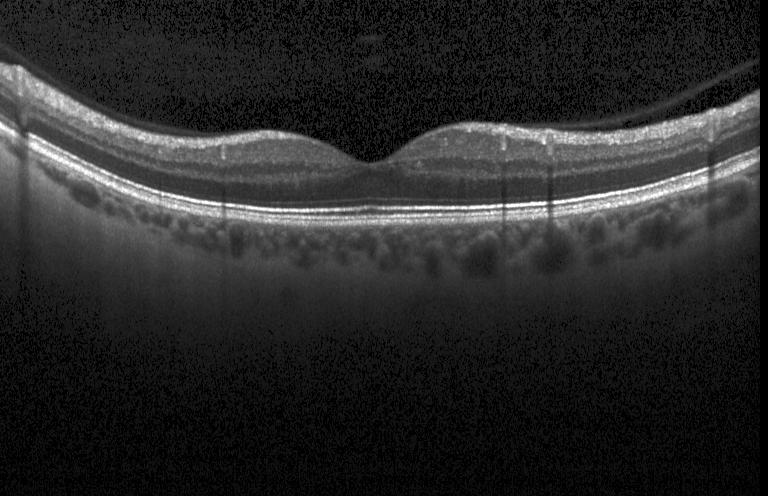

Retinal OCT cross-section showing neither CNV, DME, nor drusen.